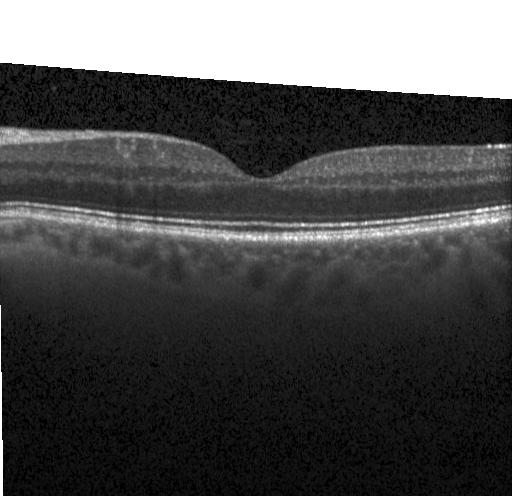

OCT line scan, macular scan, Heidelberg Spectralis OCT system, spectral-domain OCT. Macular OCT: no choroidal neovascularization, no diabetic macular edema, and no drusen.